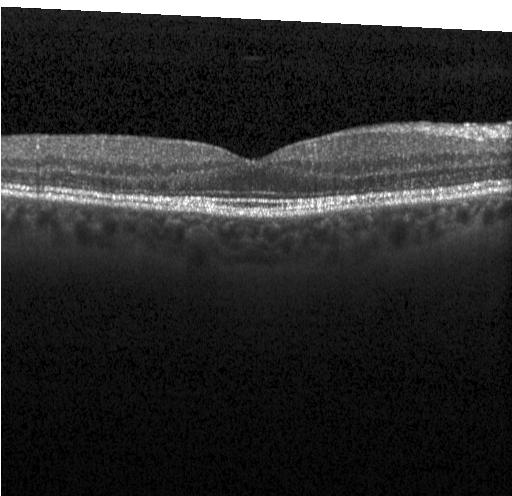

Optical coherence tomography B-scan, fovea-centered, acquired on a Heidelberg Spectralis — Impression: no choroidal neovascularization, diabetic macular edema, or drusen.